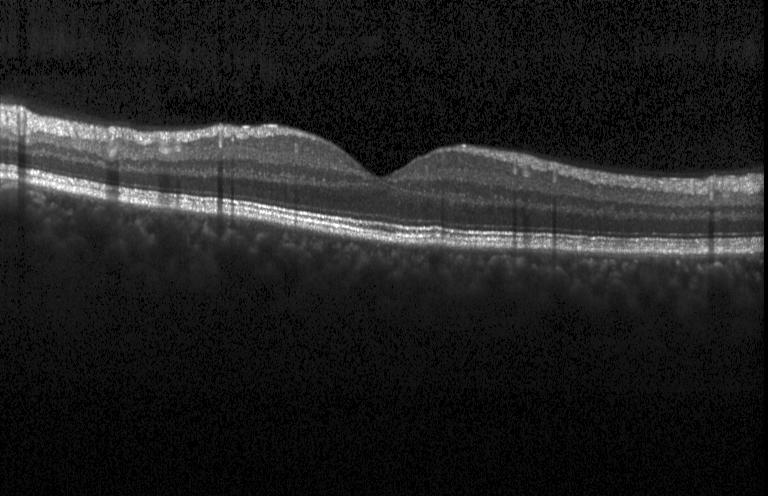

Optical coherence tomography scan. Impression: neither choroidal neovascularization, diabetic macular edema, nor drusen.